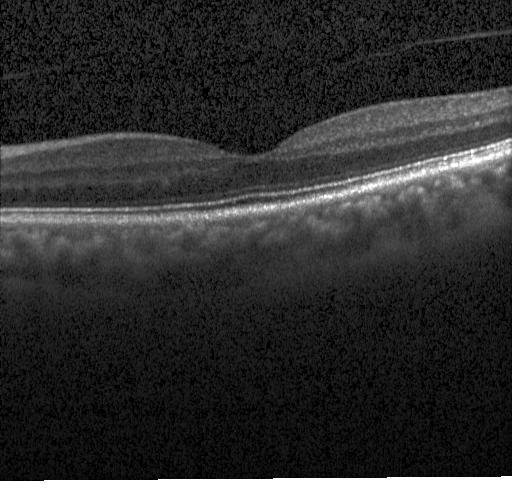 Diagnosis: no evidence of CNV, DME, or drusen.